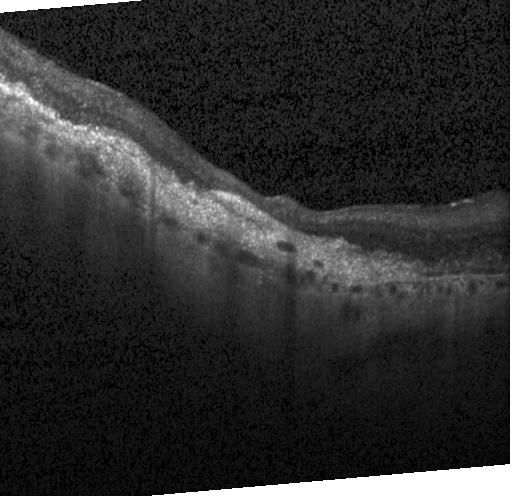
OCT finding: a choroidal neovascular membrane.